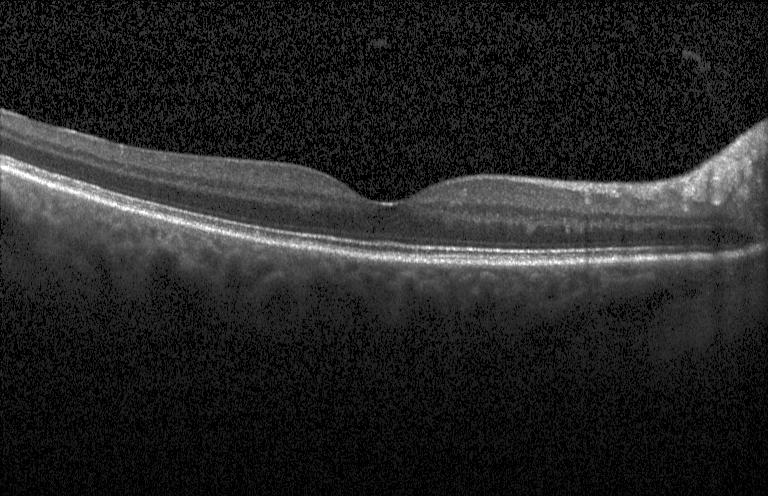 Heidelberg Spectralis OCT system; centered on the fovea; retinal OCT cross-section; SD-OCT.
The scan shows no evidence of choroidal neovascularization, diabetic macular edema, or drusen.